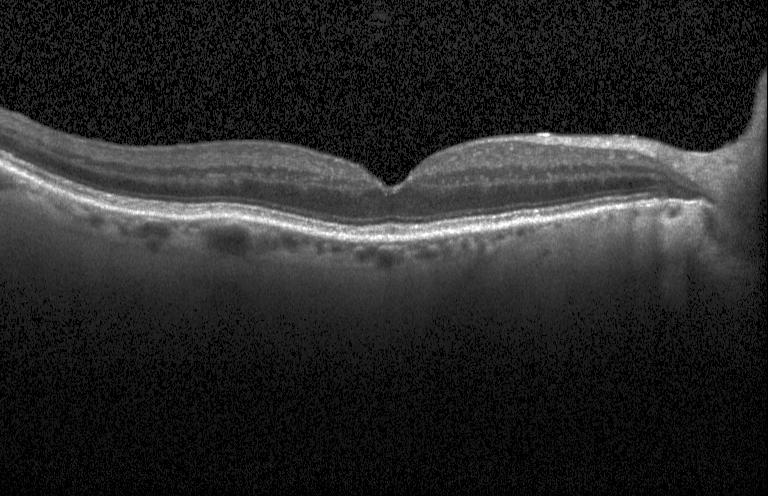 Horizontal scan through the fovea · spectral-domain optical coherence tomography · OCT B-scan · acquired on a Heidelberg Spectralis
Macular OCT: no evidence of choroidal neovascularization, diabetic macular edema, or drusen.